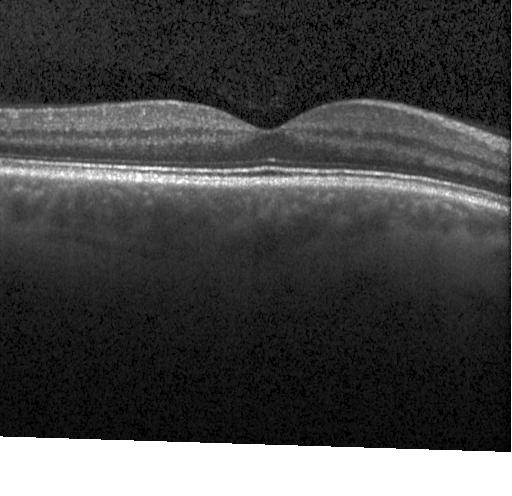

Instrument: Heidelberg Spectralis; retinal OCT cross-section; horizontal scan through the fovea — No choroidal neovascularization, no diabetic macular edema, and no drusen.